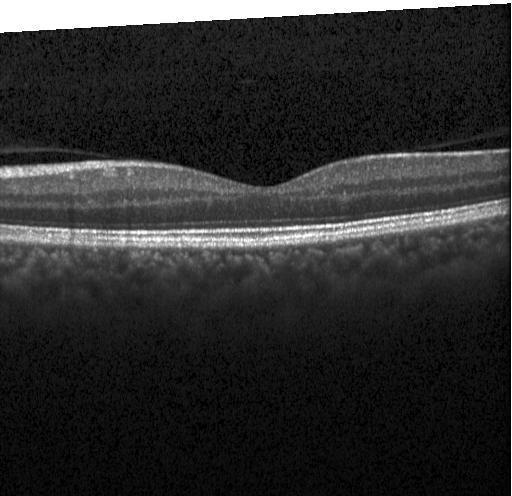

Optical coherence tomography B-scan. Macular scan. Spectral-domain optical coherence tomography — Diagnosis: neither choroidal neovascularization, diabetic macular edema, nor drusen.